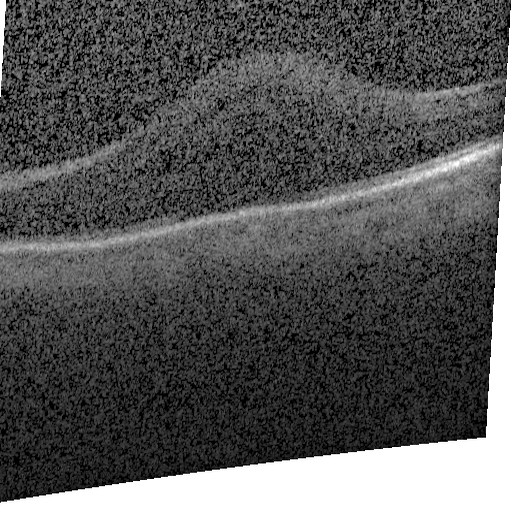

OCT B-scan; instrument: Heidelberg Spectralis; through the macula.
Impression: diabetic macular edema.